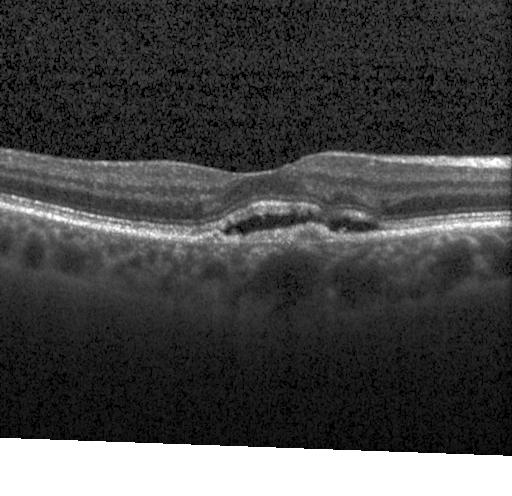

This B-scan demonstrates a choroidal neovascular membrane.